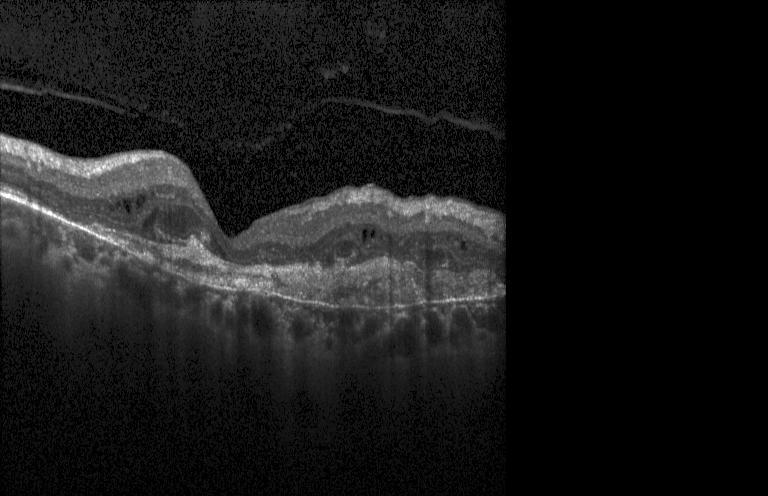
Spectral-domain OCT, fovea-centered, retinal OCT cross-section. Finding: choroidal neovascularization (CNV).